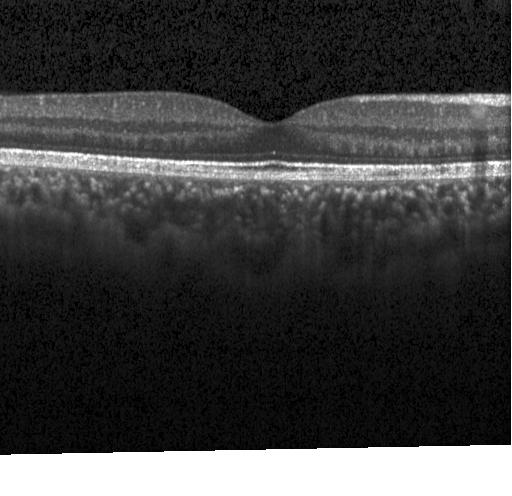
Horizontal scan through the fovea; retinal OCT B-scan; spectral-domain optical coherence tomography.
Diagnosis: no CNV, no DME, and no drusen.